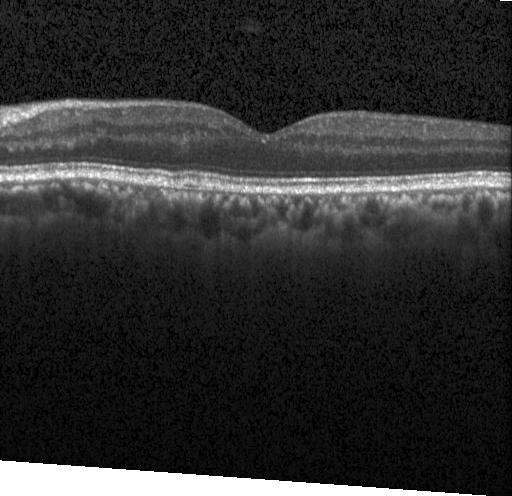
Retinal OCT B-scan — No evidence of choroidal neovascularization, diabetic macular edema, or drusen.